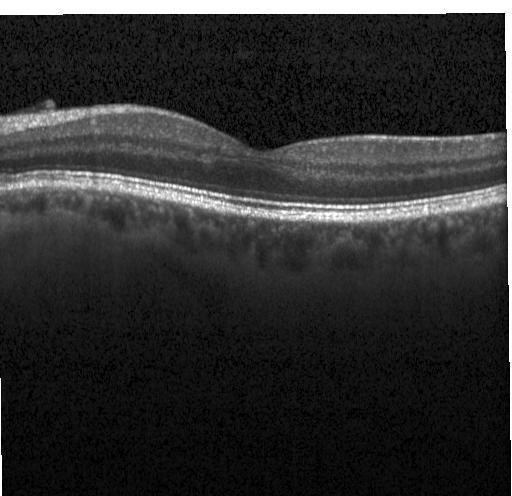 OCT B-scan showing no choroidal neovascularization, diabetic macular edema, or drusen.